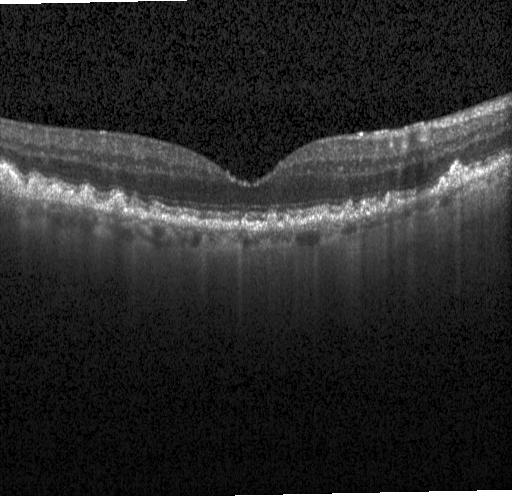
Through the macula · retinal OCT B-scan.
Sub-RPE drusenoid deposits.